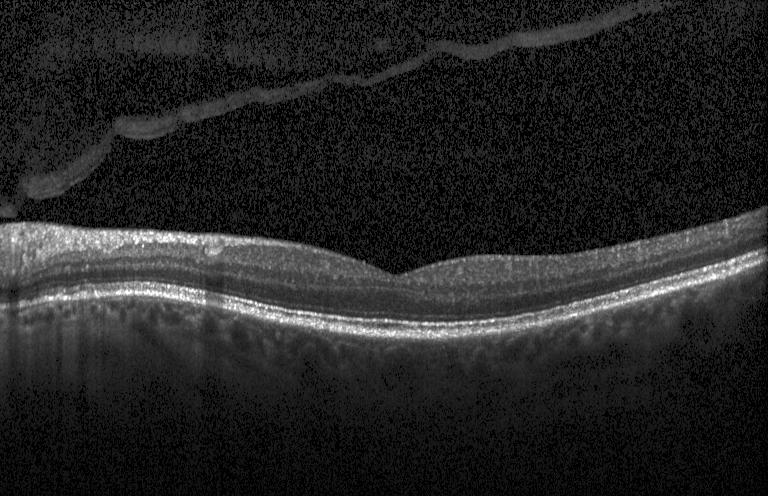
Dx: no choroidal neovascularization, diabetic macular edema, or drusen.